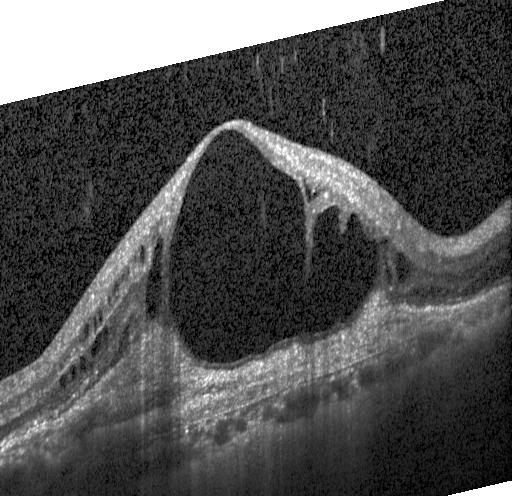
OCT B-scan showing a choroidal neovascular membrane.